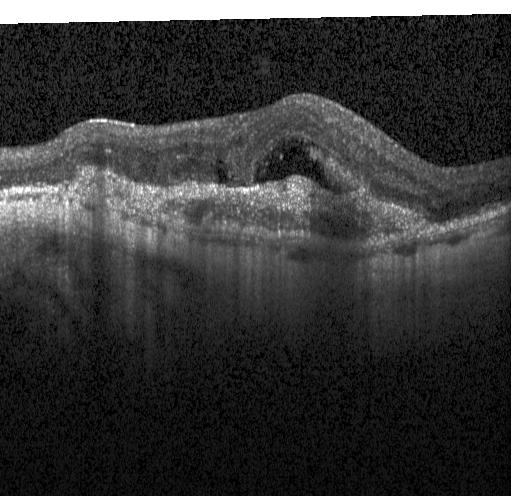 Retinal OCT cross-section showing CNV.